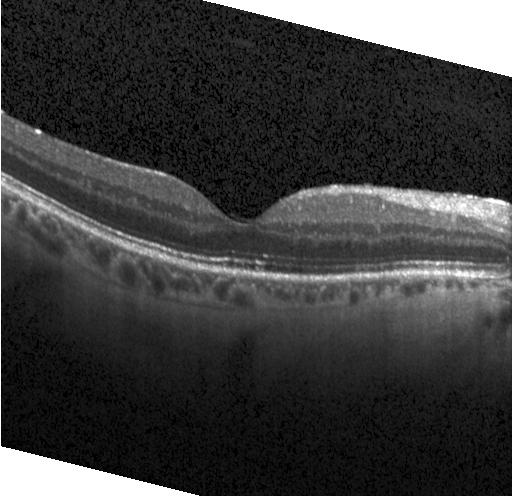

Heidelberg Spectralis OCT system. Centered on the fovea. OCT line scan. The scan shows no choroidal neovascularization, no diabetic macular edema, and no drusen.